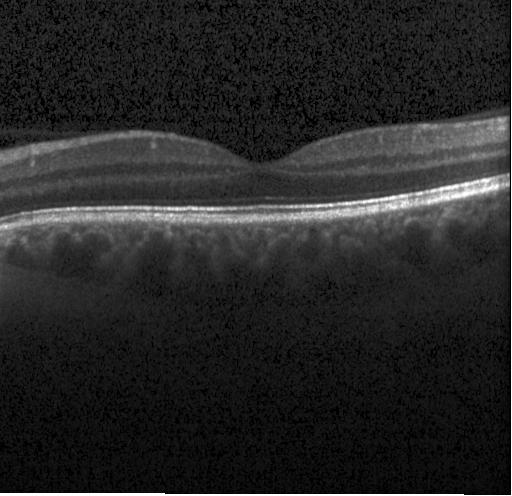

Horizontal scan through the fovea. Optical coherence tomography B-scan. SD-OCT. Instrument: Heidelberg Spectralis — This B-scan demonstrates no CNV, no DME, and no drusen.